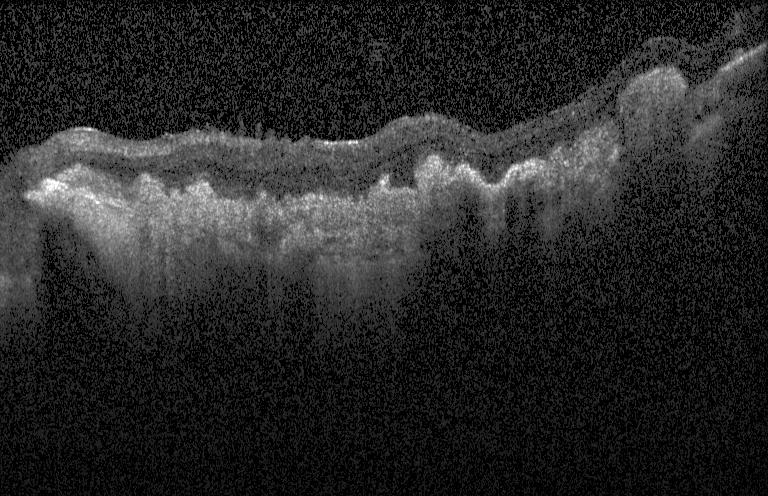

Spectral-domain optical coherence tomography · retinal OCT B-scan
This B-scan demonstrates choroidal neovascularization.